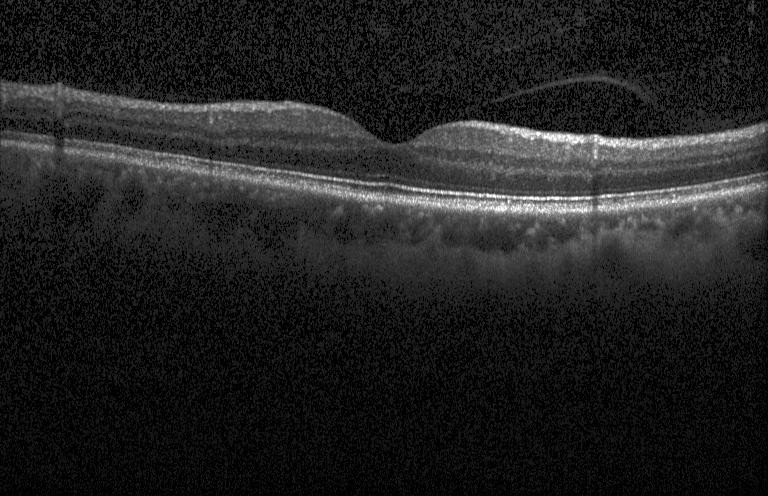

OCT line scan
Finding: no evidence of choroidal neovascularization, diabetic macular edema, or drusen.